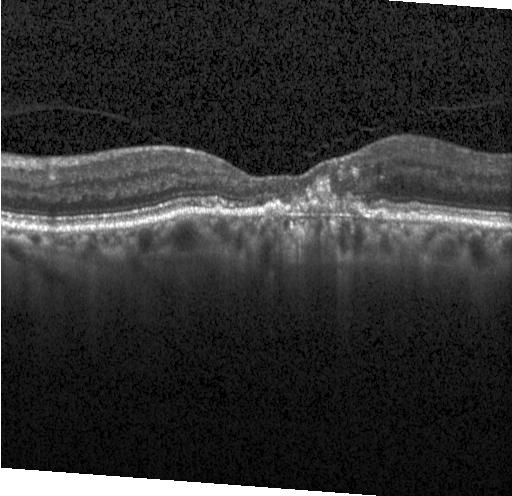 SD-OCT. Fovea-centered. OCT line scan. Choroidal neovascularization (CNV).